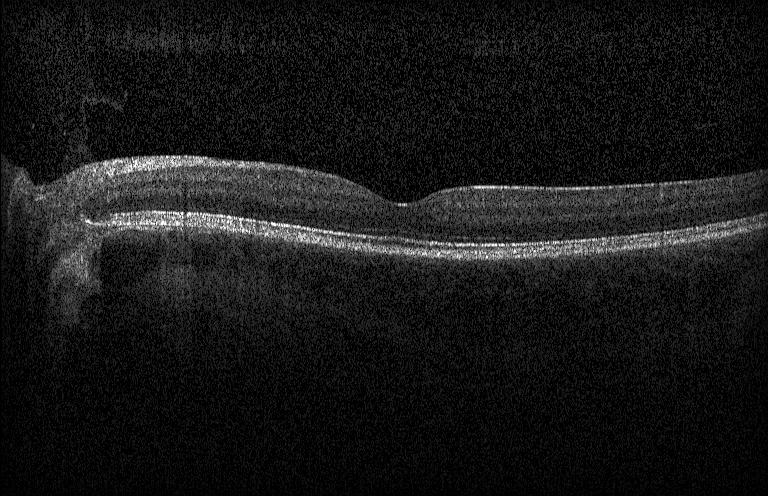 Optical coherence tomography B-scan; through the macula; spectral-domain OCT — OCT finding: neither CNV, DME, nor drusen.